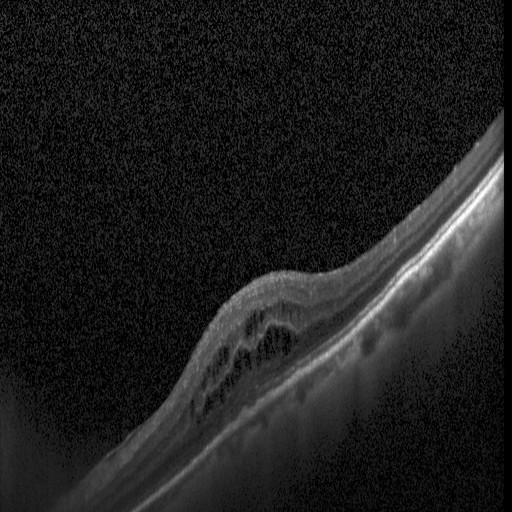

Impression: diabetic macular edema.